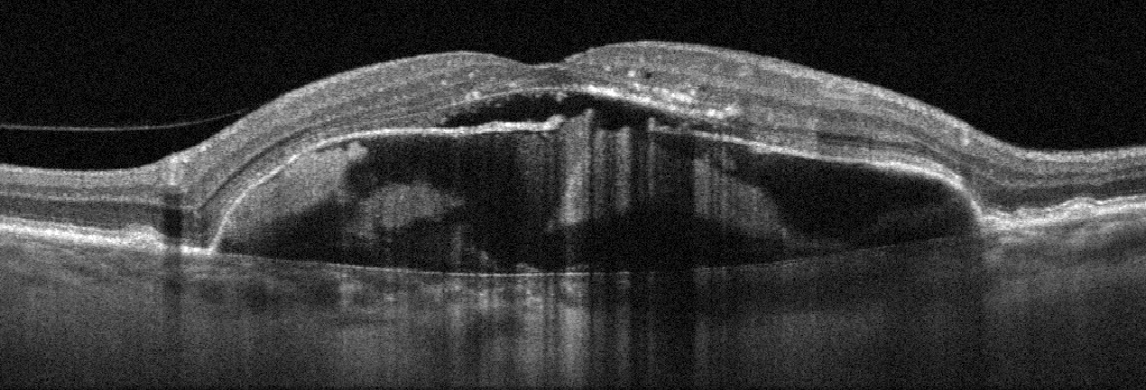
The scan shows AMD.